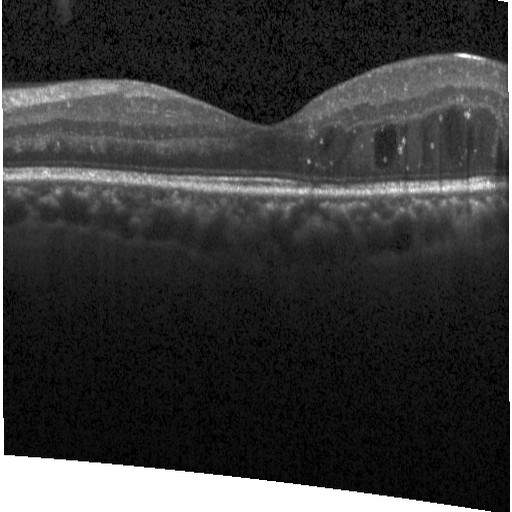
Optical coherence tomography scan.
Assessment: DME.